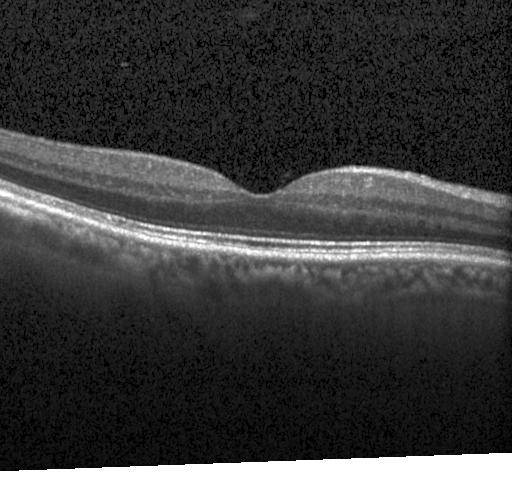
Optical coherence tomography scan — The scan shows neither choroidal neovascularization, diabetic macular edema, nor drusen.